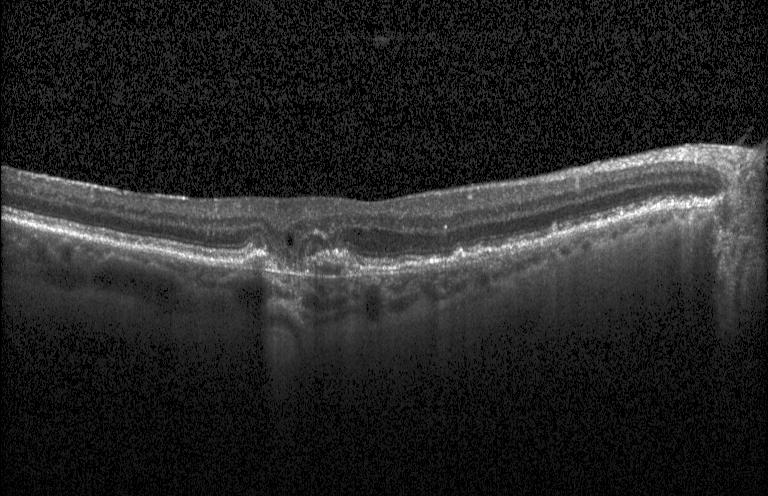 The scan shows choroidal neovascularization.